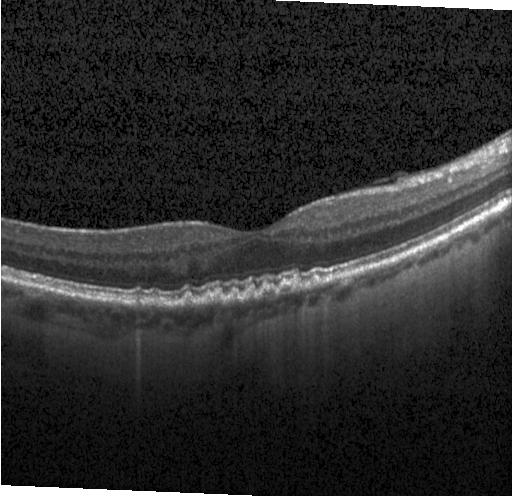

SD-OCT. Fovea-centered. Retinal OCT B-scan — Assessment: drusen.